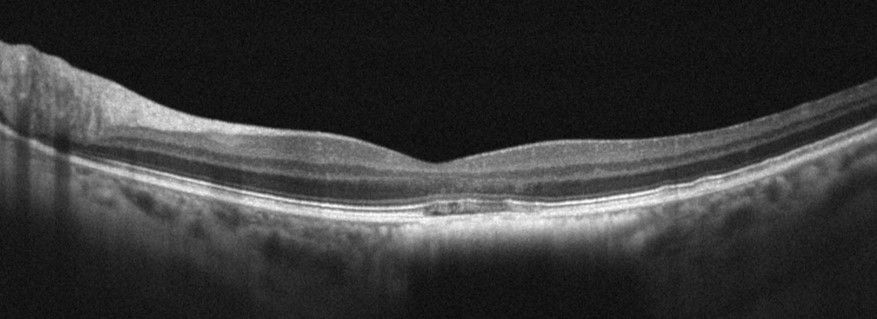 Macular OCT demonstrating AMD.